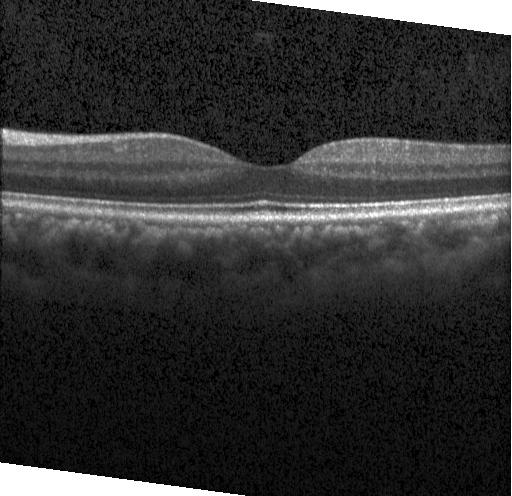 OCT B-scan — Macular OCT: no choroidal neovascularization, diabetic macular edema, or drusen.